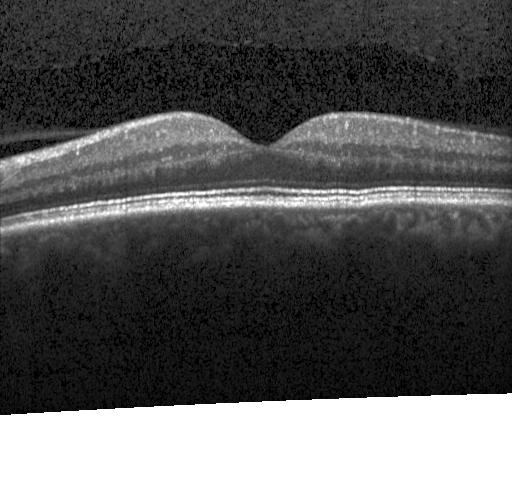
Retinal OCT B-scan; spectral-domain optical coherence tomography. Assessment: no choroidal neovascularization, diabetic macular edema, or drusen.